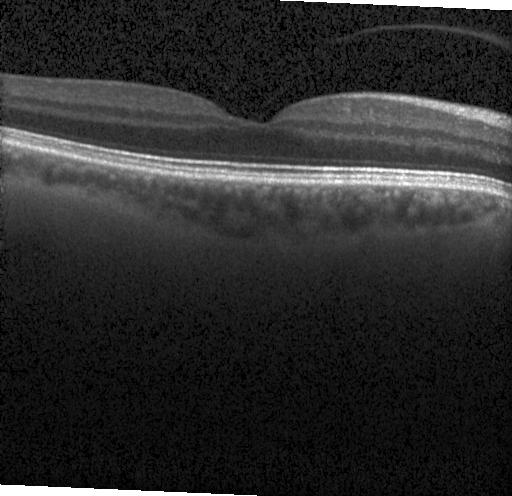 Optical coherence tomography B-scan — This B-scan demonstrates neither CNV, DME, nor drusen.